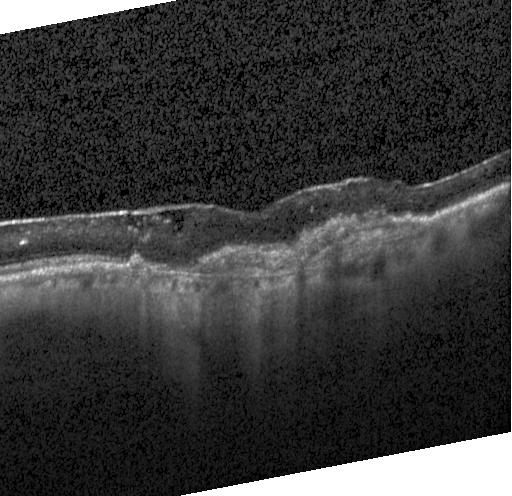

Heidelberg Spectralis · OCT B-scan.
Diagnosis: choroidal neovascularization.